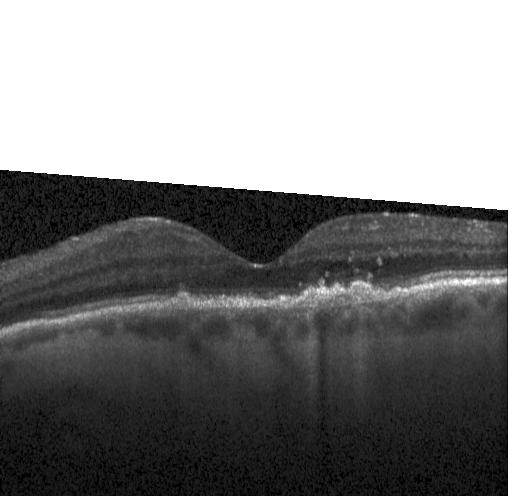
Retinal OCT cross-section showing sub-RPE drusenoid deposits.